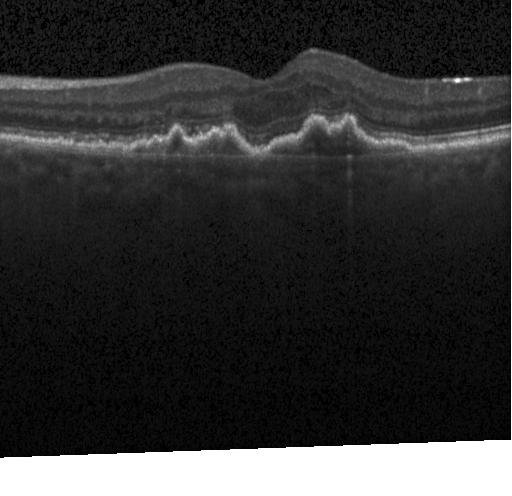 OCT B-scan. Spectral-domain optical coherence tomography. Macular scan. Heidelberg Spectralis — This B-scan demonstrates a choroidal neovascular membrane.